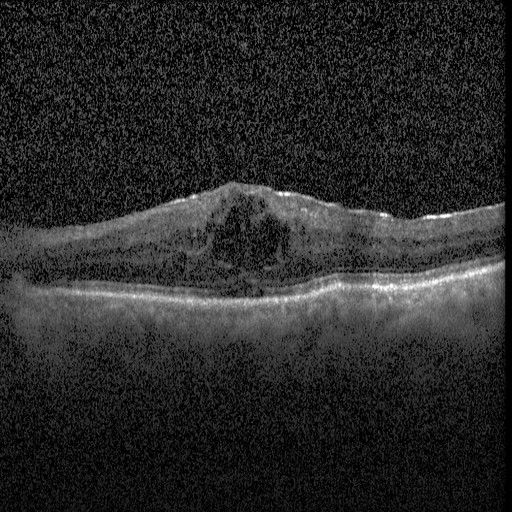 OCT B-scan showing diabetic macular edema (DME).